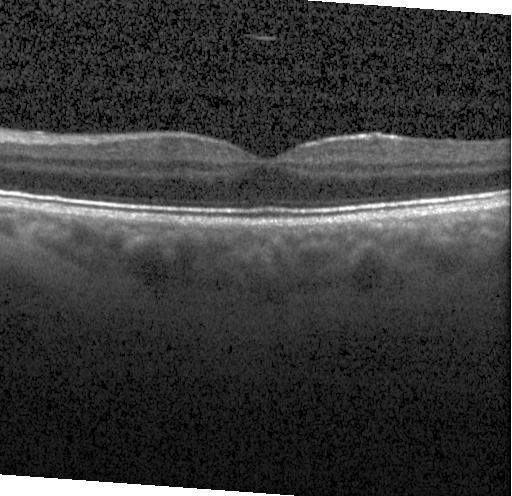 Optical coherence tomography B-scan · spectral-domain optical coherence tomography
Impression: neither choroidal neovascularization, diabetic macular edema, nor drusen.